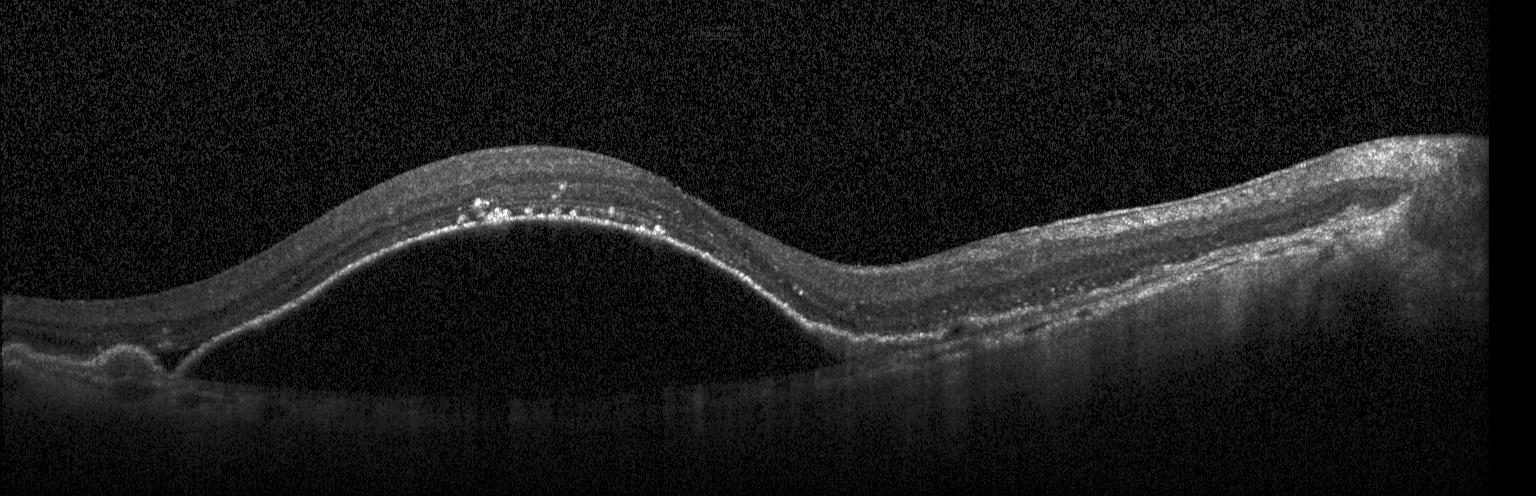

Spectral-domain OCT; through the macula; retinal OCT B-scan; Heidelberg Spectralis
Choroidal neovascularization.